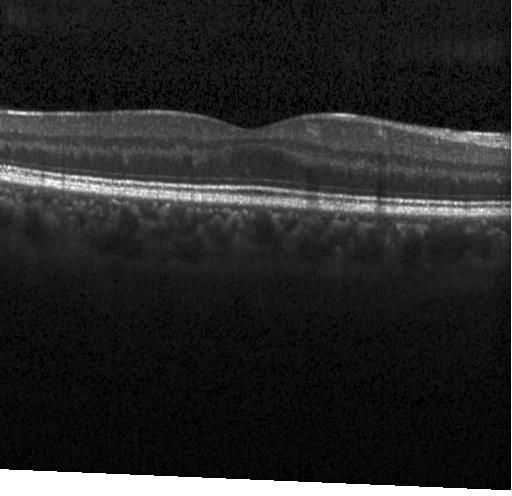 Diagnosis: no choroidal neovascularization, diabetic macular edema, or drusen.